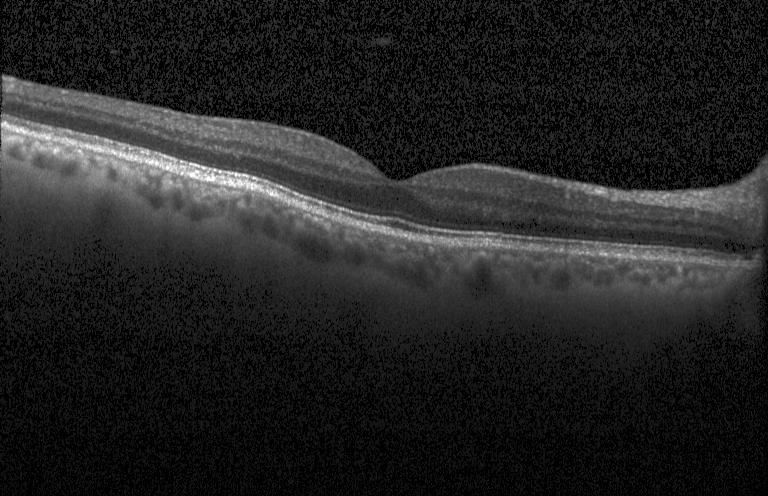
Finding: no choroidal neovascularization, diabetic macular edema, or drusen.